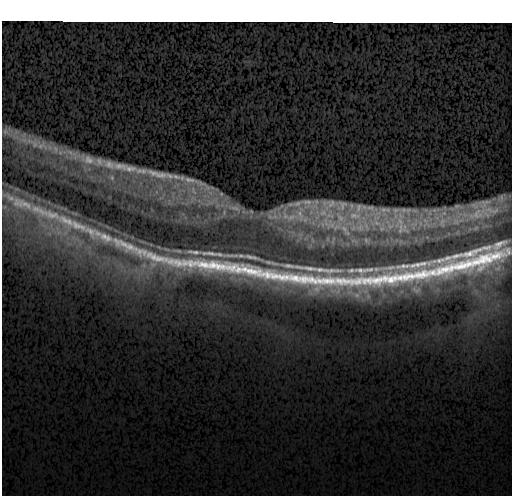

Centered on the fovea · OCT B-scan · SD-OCT · Heidelberg Spectralis OCT system. This B-scan demonstrates no CNV, DME, or drusen.